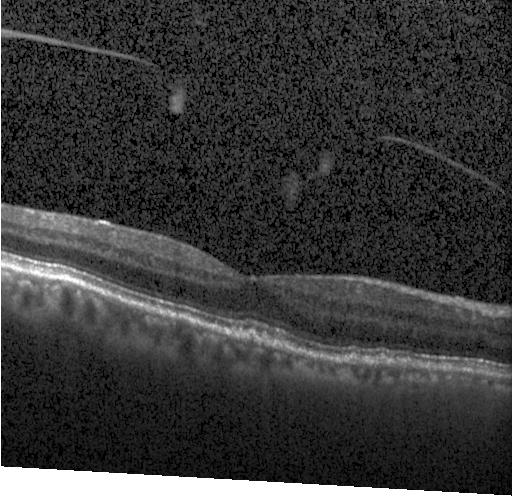
Macular scan. Retinal OCT B-scan
Finding: drusen.